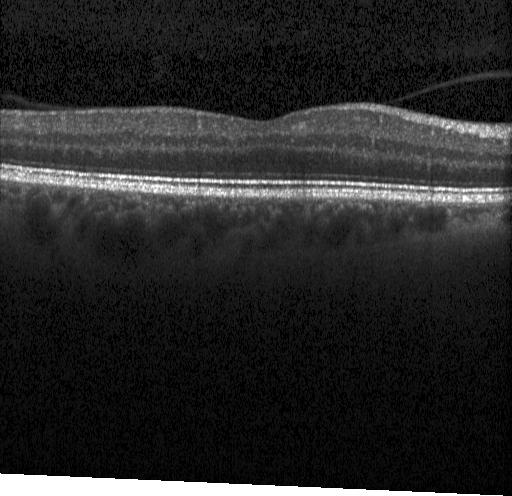
Retinal OCT B-scan.
Impression: no choroidal neovascularization, no diabetic macular edema, and no drusen.